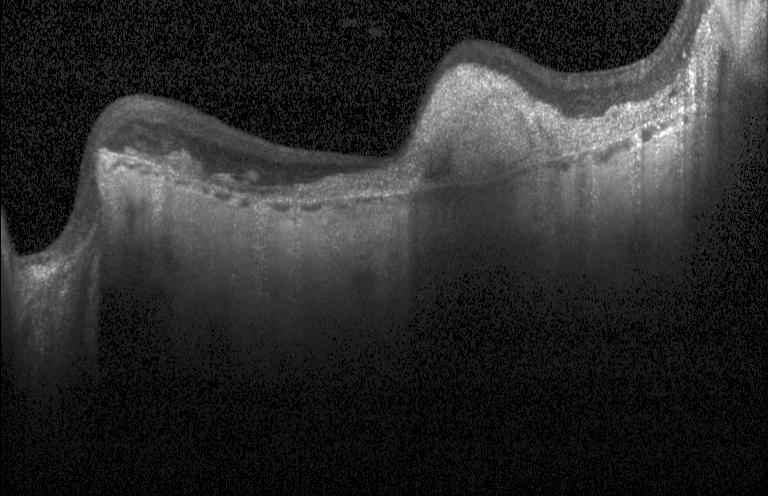
This B-scan demonstrates choroidal neovascularization (CNV).